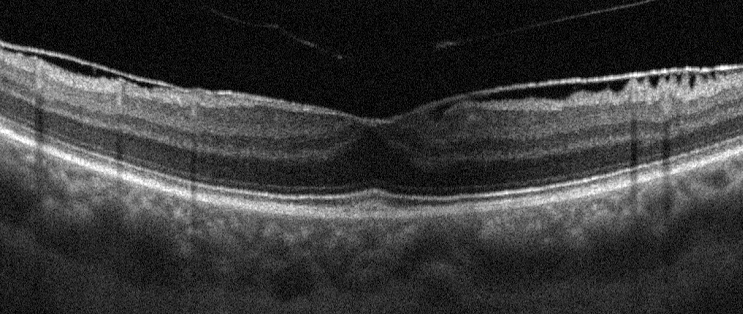 Instrument: Optovue Avanti RTVue XR, optical coherence tomography B-scan — This B-scan demonstrates ERM.